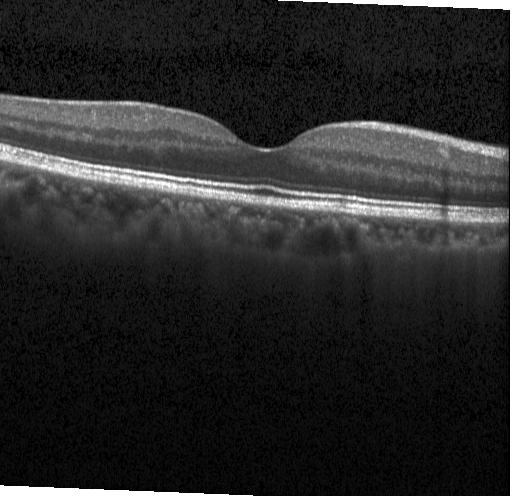 Diagnosis: no choroidal neovascularization, diabetic macular edema, or drusen.